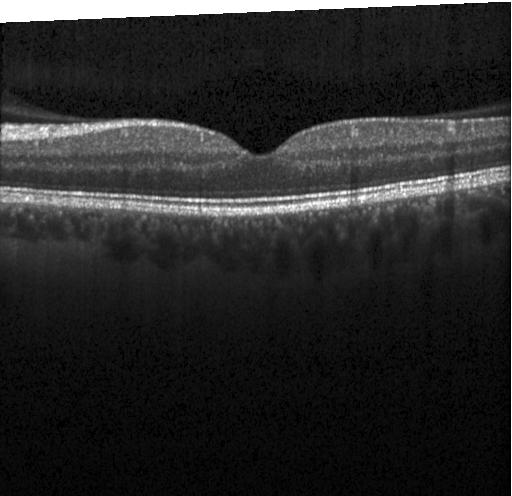

OCT scan showing no CNV, no DME, and no drusen.